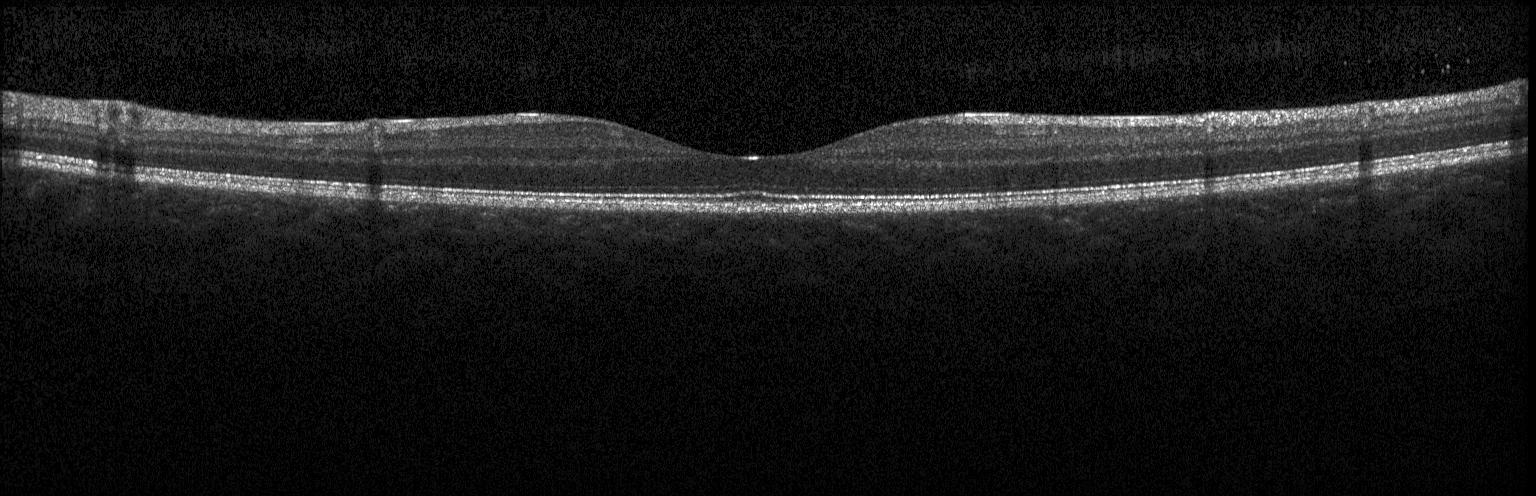 Optical coherence tomography scan
Diagnosis: no choroidal neovascularization, diabetic macular edema, or drusen.